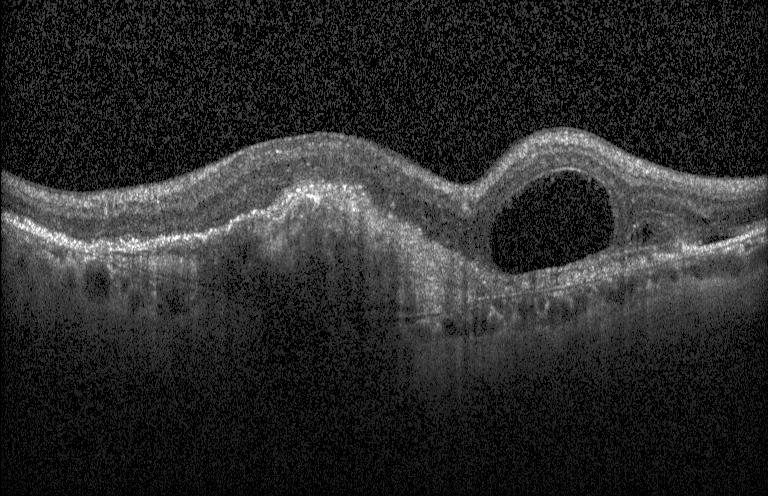
Diagnosis: a choroidal neovascular membrane.